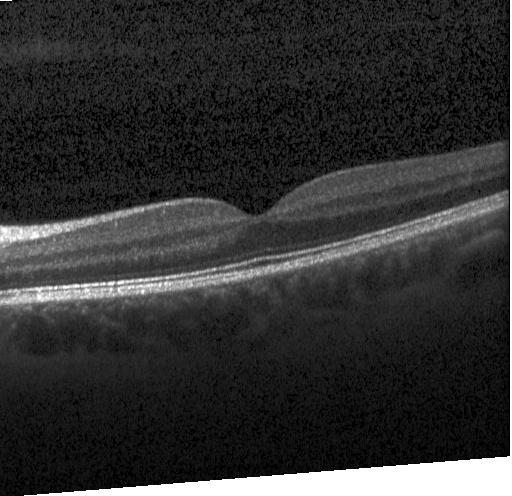

Spectral-domain OCT. Heidelberg Spectralis OCT system. OCT B-scan — Finding: no evidence of choroidal neovascularization, diabetic macular edema, or drusen.